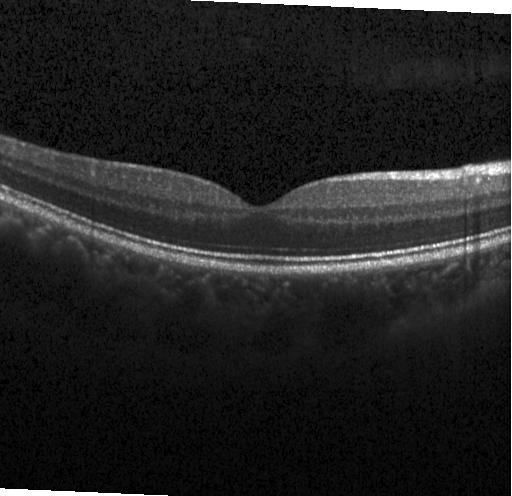 Impression: no evidence of choroidal neovascularization, diabetic macular edema, or drusen.